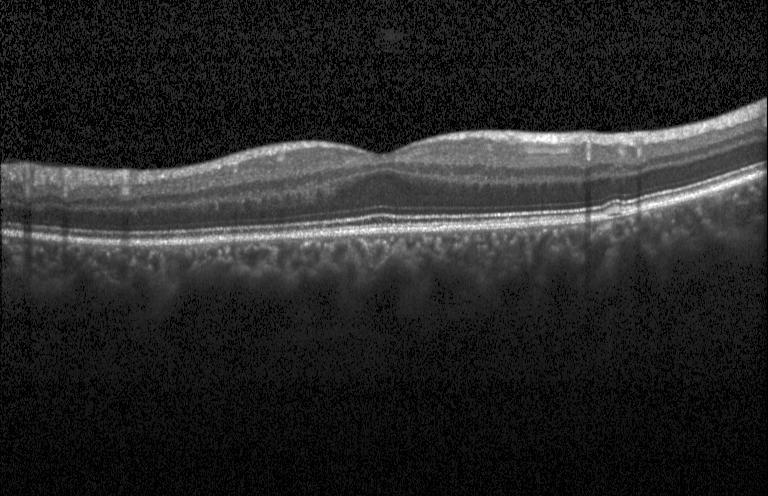
Dx: no evidence of choroidal neovascularization, diabetic macular edema, or drusen.